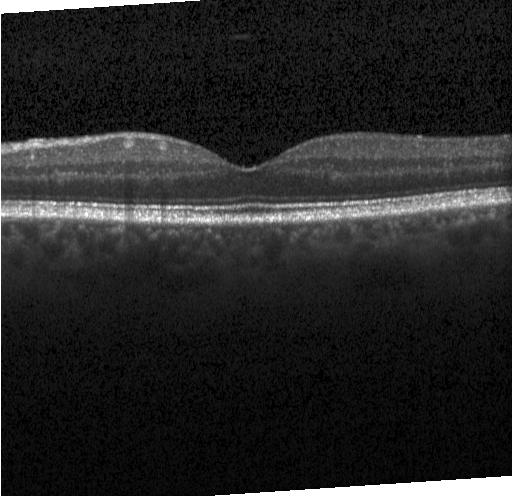 Diagnosis: no choroidal neovascularization, diabetic macular edema, or drusen.